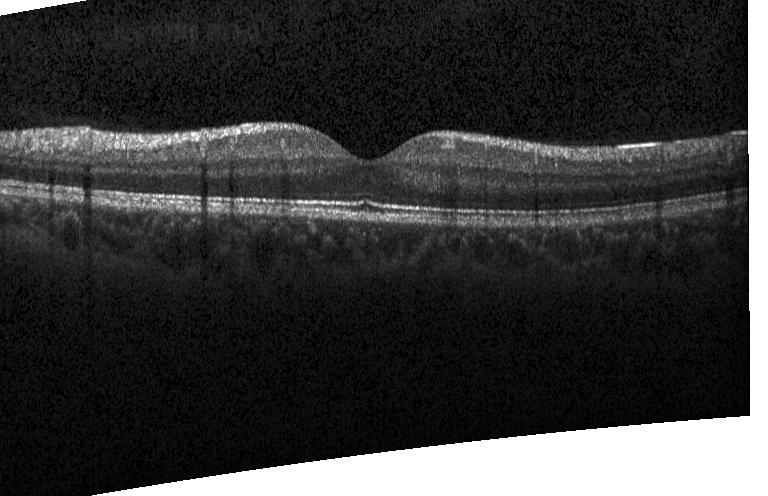

Assessment: no choroidal neovascularization, diabetic macular edema, or drusen.